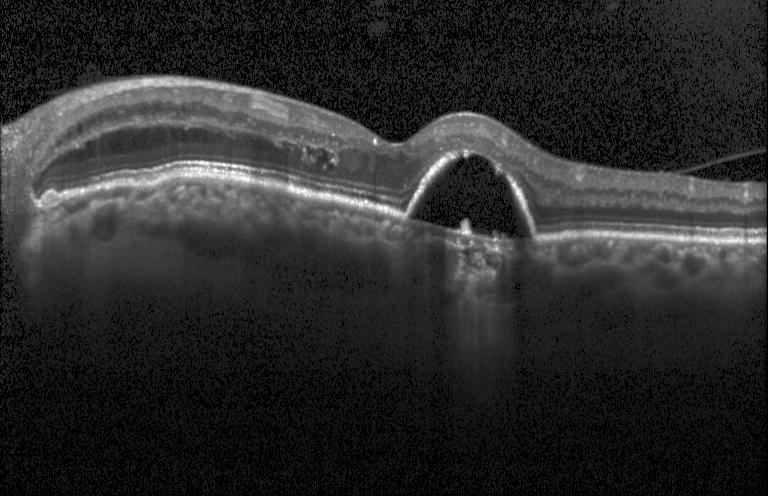 Diagnosis: choroidal neovascularization (CNV).